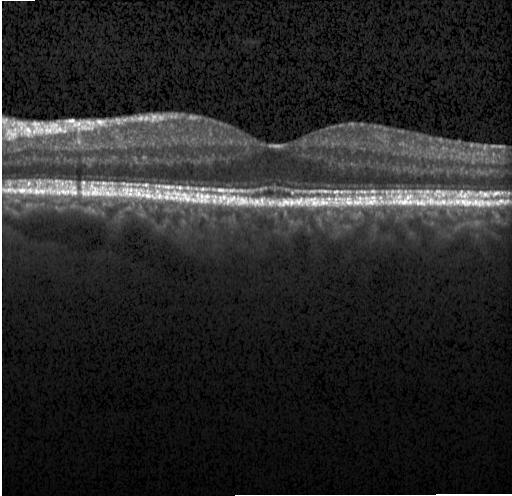
Macular scan; optical coherence tomography scan
OCT finding: no choroidal neovascularization, no diabetic macular edema, and no drusen.